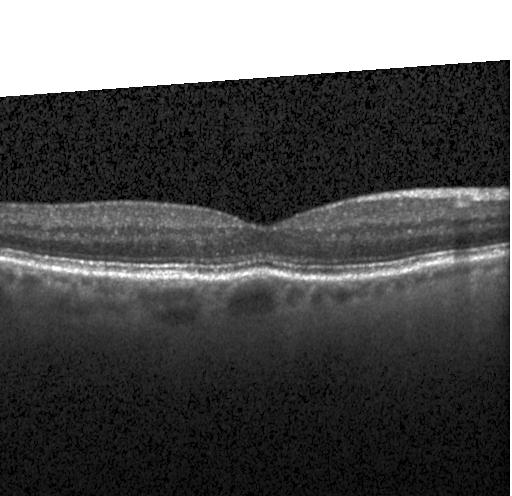

Heidelberg Spectralis OCT system. Spectral-domain OCT. Fovea-centered. Retinal OCT cross-section.
Finding: no evidence of choroidal neovascularization, diabetic macular edema, or drusen.